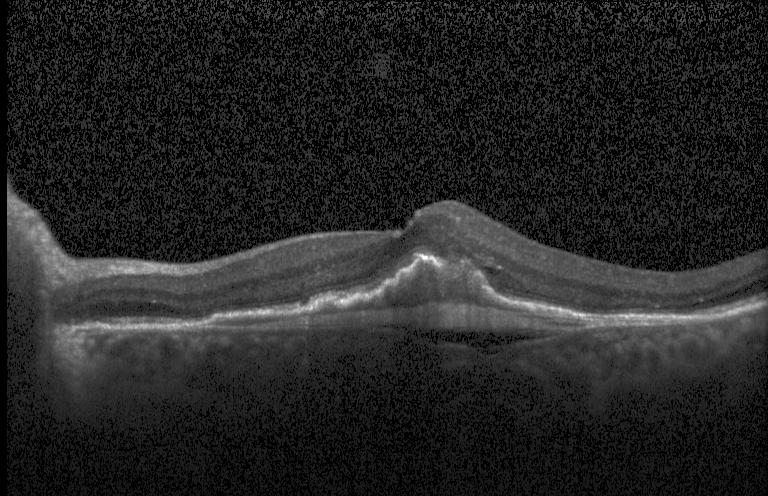

OCT B-scan — Impression: a choroidal neovascular membrane.